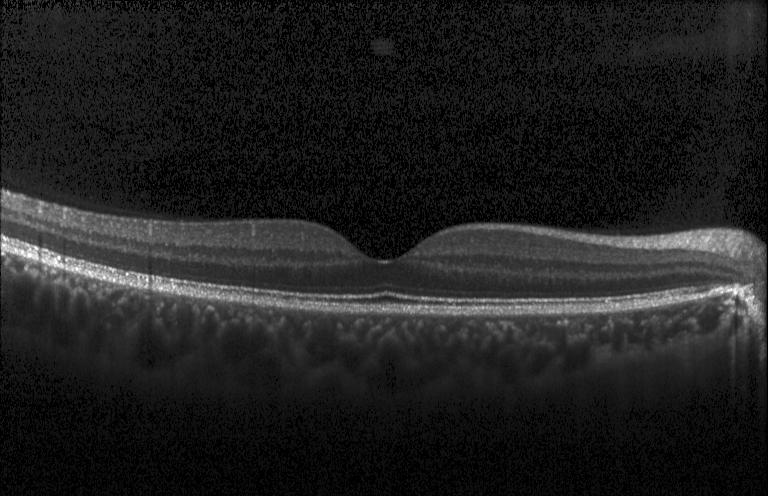
Retinal OCT B-scan — Dx: no evidence of CNV, DME, or drusen.